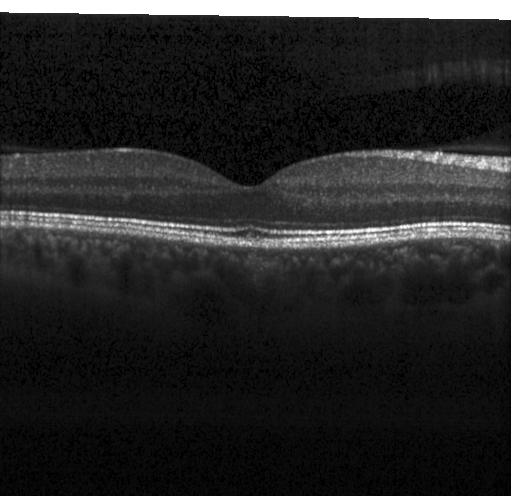 Optical coherence tomography scan.
Impression: no evidence of choroidal neovascularization, diabetic macular edema, or drusen.